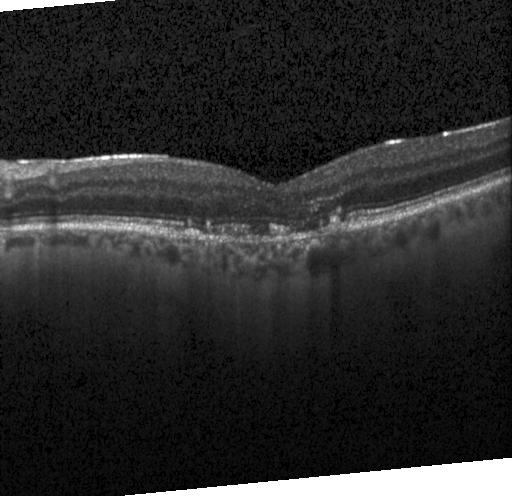 Finding: choroidal neovascularization (CNV).